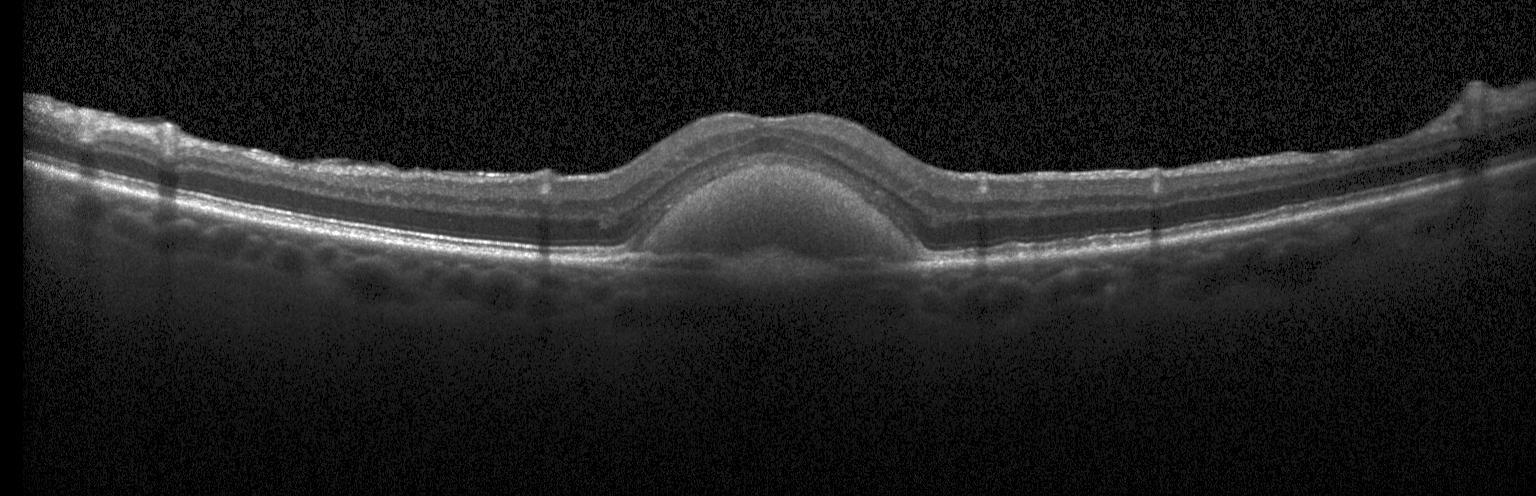 Finding: a choroidal neovascular membrane.